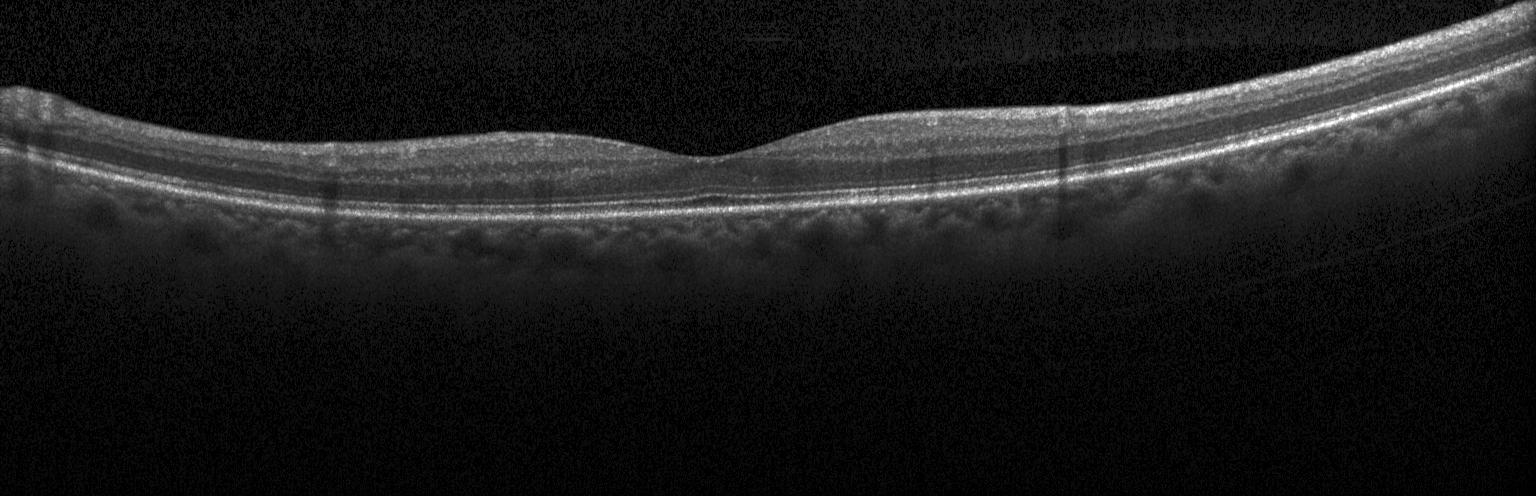

SD-OCT · horizontal scan through the fovea · retinal OCT B-scan · acquired on a Heidelberg Spectralis — Diagnosis: no choroidal neovascularization, no diabetic macular edema, and no drusen.